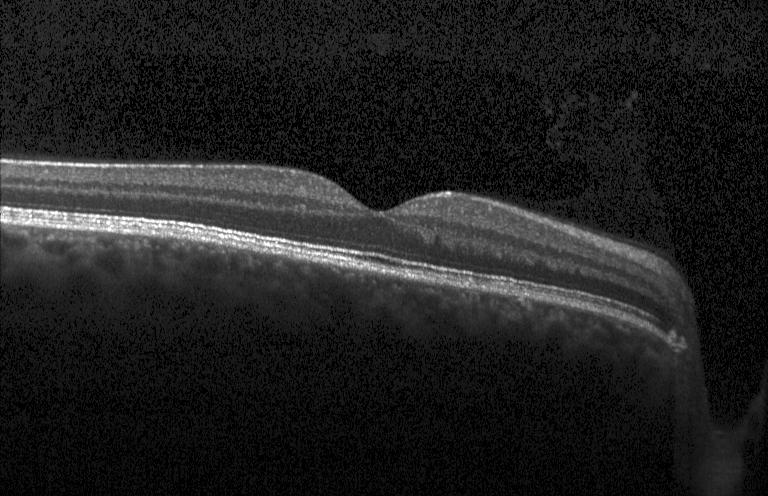

This B-scan demonstrates neither CNV, DME, nor drusen.